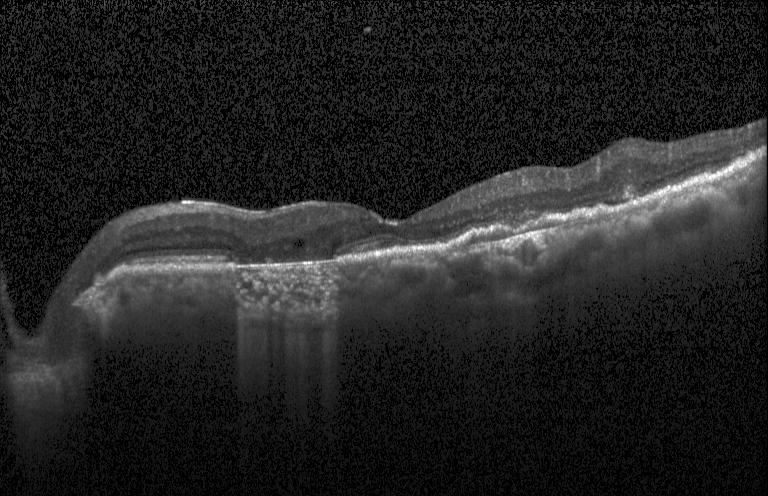 OCT finding: choroidal neovascularization (CNV).